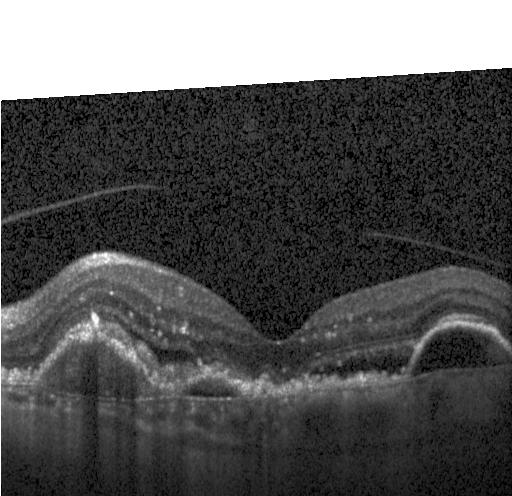

Fovea-centered, retinal OCT B-scan, SD-OCT, Heidelberg Spectralis.
Finding: choroidal neovascularization.